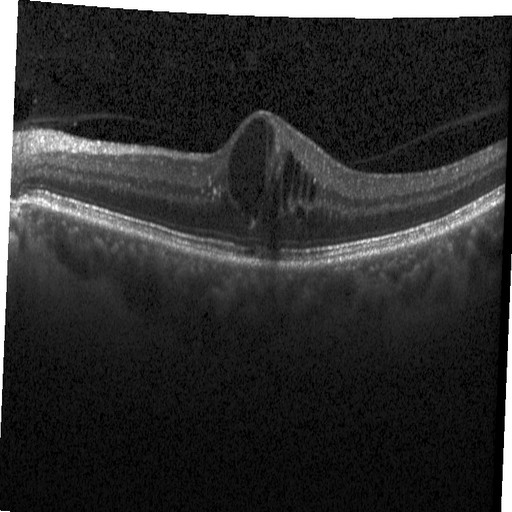
Impression: DME.